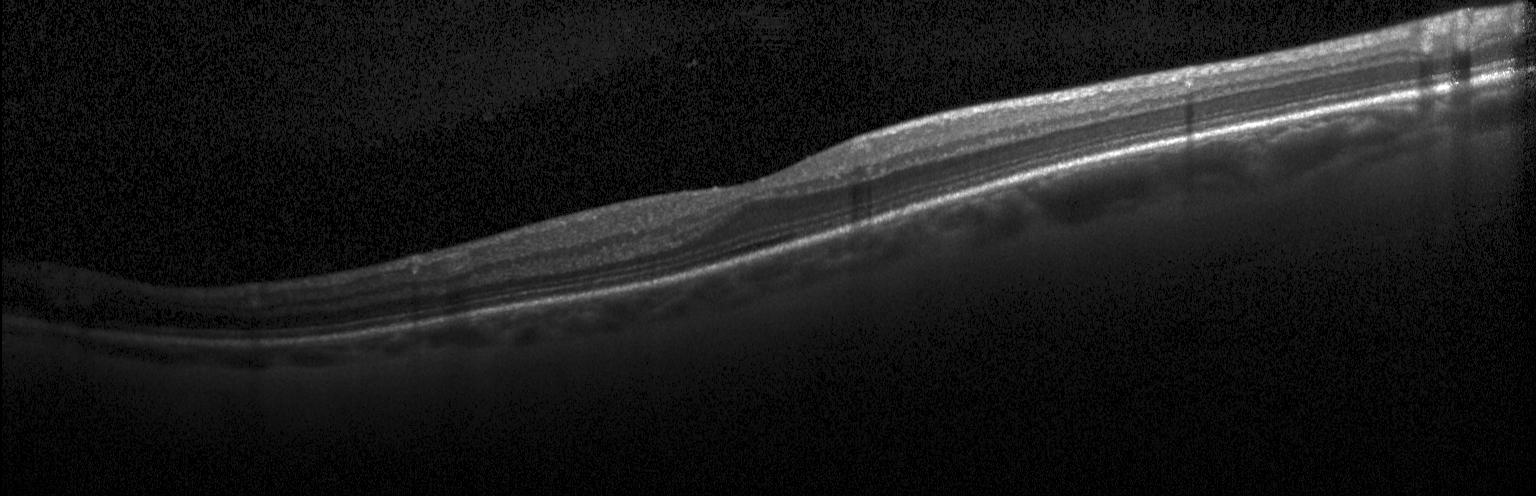 Retinal OCT cross-section. Through the macula.
Impression: no evidence of choroidal neovascularization, diabetic macular edema, or drusen.